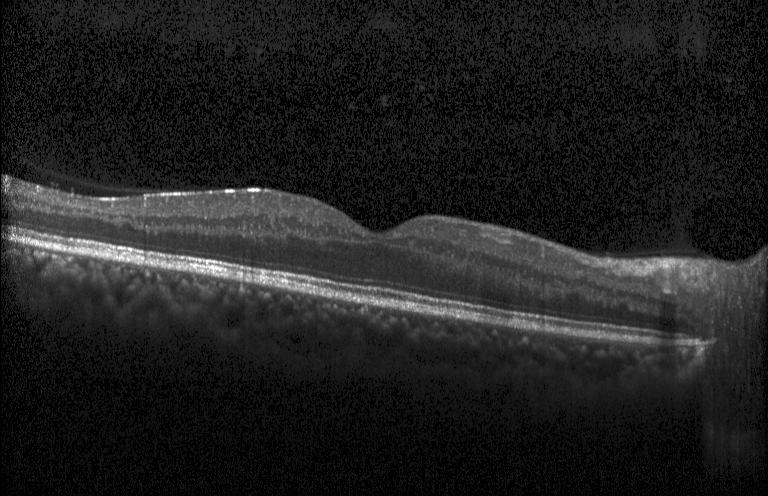 Through the macula · spectral-domain optical coherence tomography · retinal OCT cross-section.
Finding: no evidence of choroidal neovascularization, diabetic macular edema, or drusen.